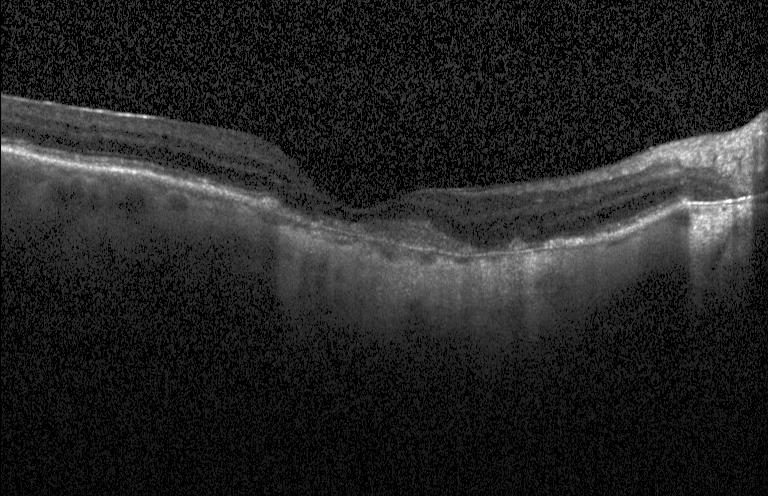

Instrument: Heidelberg Spectralis; retinal OCT B-scan; macular scan; SD-OCT.
OCT finding: a choroidal neovascular membrane.